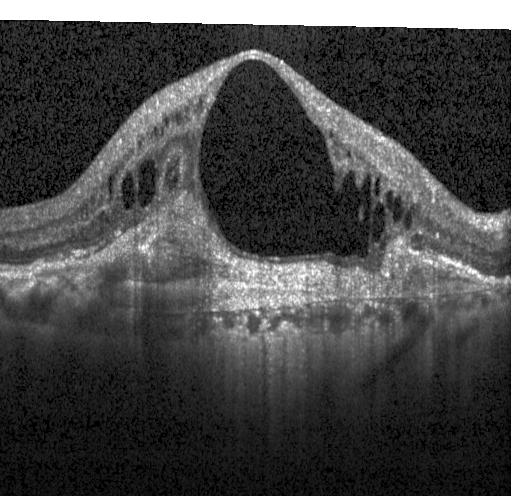

Macular OCT demonstrating choroidal neovascularization.